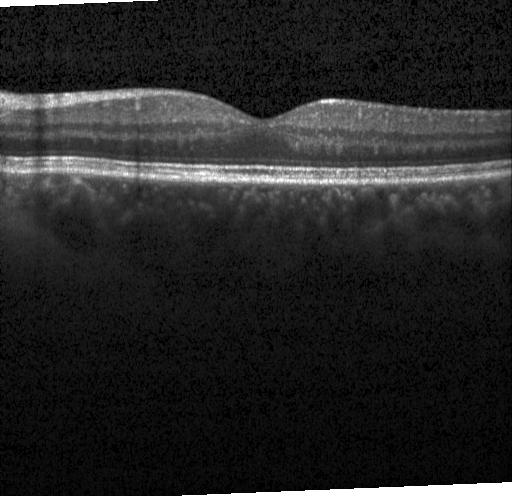

Optical coherence tomography scan, SD-OCT, horizontal scan through the fovea. The scan shows neither choroidal neovascularization, diabetic macular edema, nor drusen.